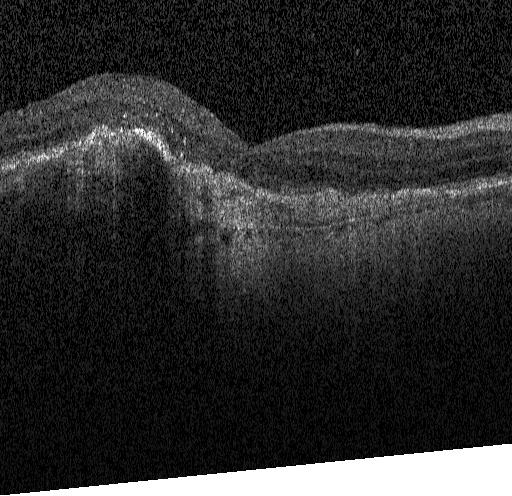

Optical coherence tomography scan; centered on the fovea.
Assessment: choroidal neovascularization.